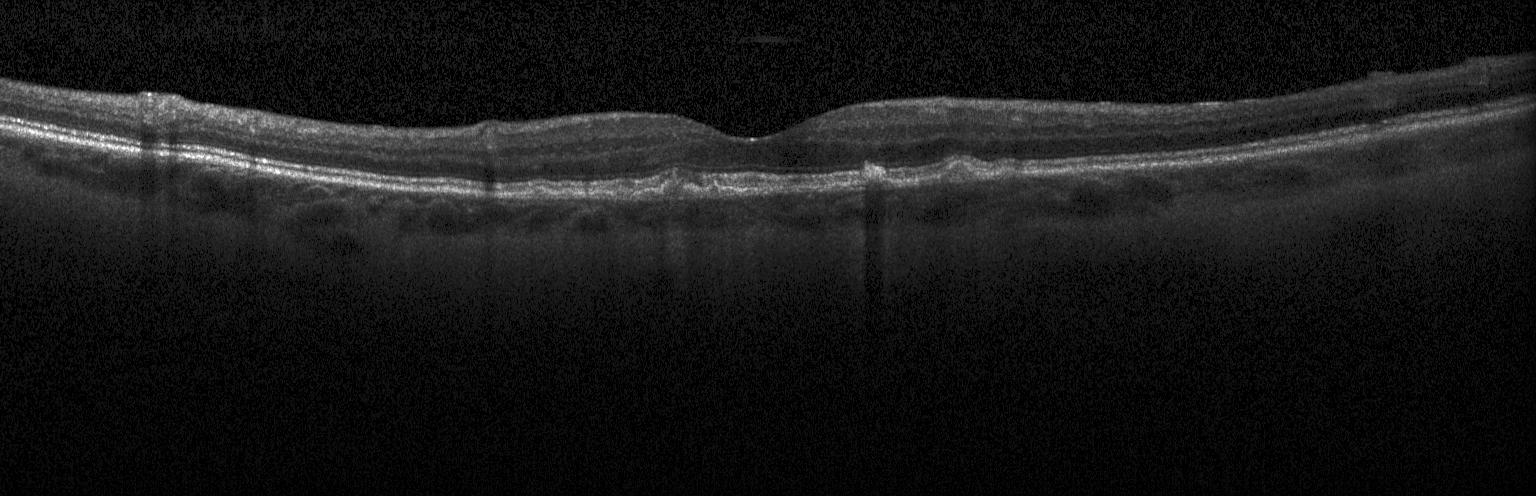 Retinal OCT cross-section showing multiple drusen.